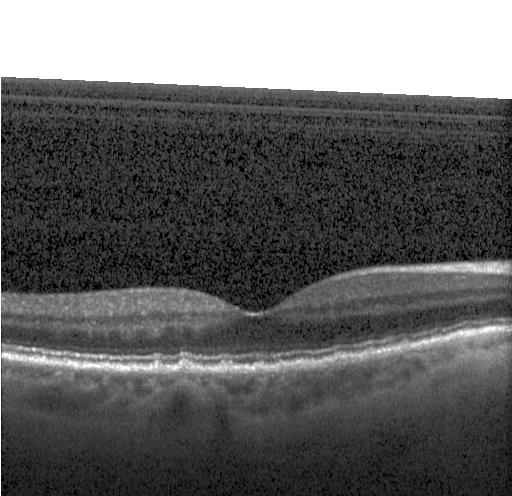
Horizontal scan through the fovea · OCT B-scan — This B-scan demonstrates sub-RPE drusenoid deposits.